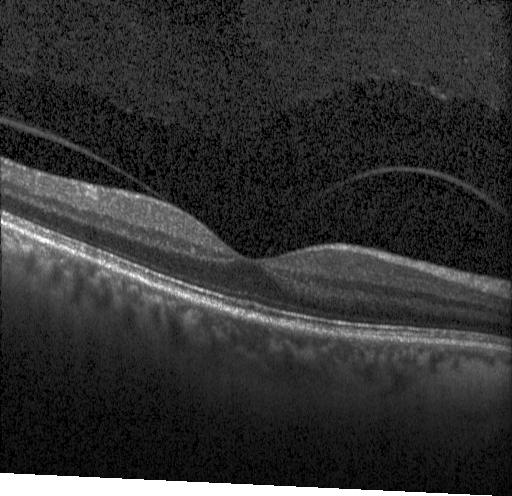
Impression: no choroidal neovascularization, diabetic macular edema, or drusen.